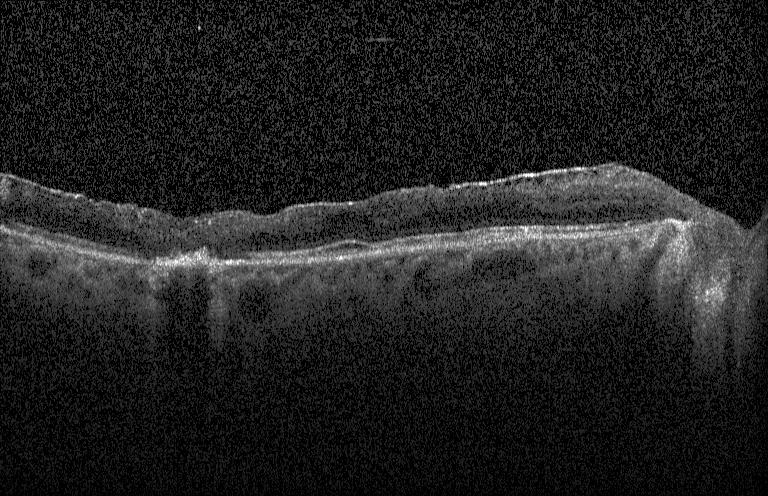
Diagnosis: choroidal neovascularization (CNV).